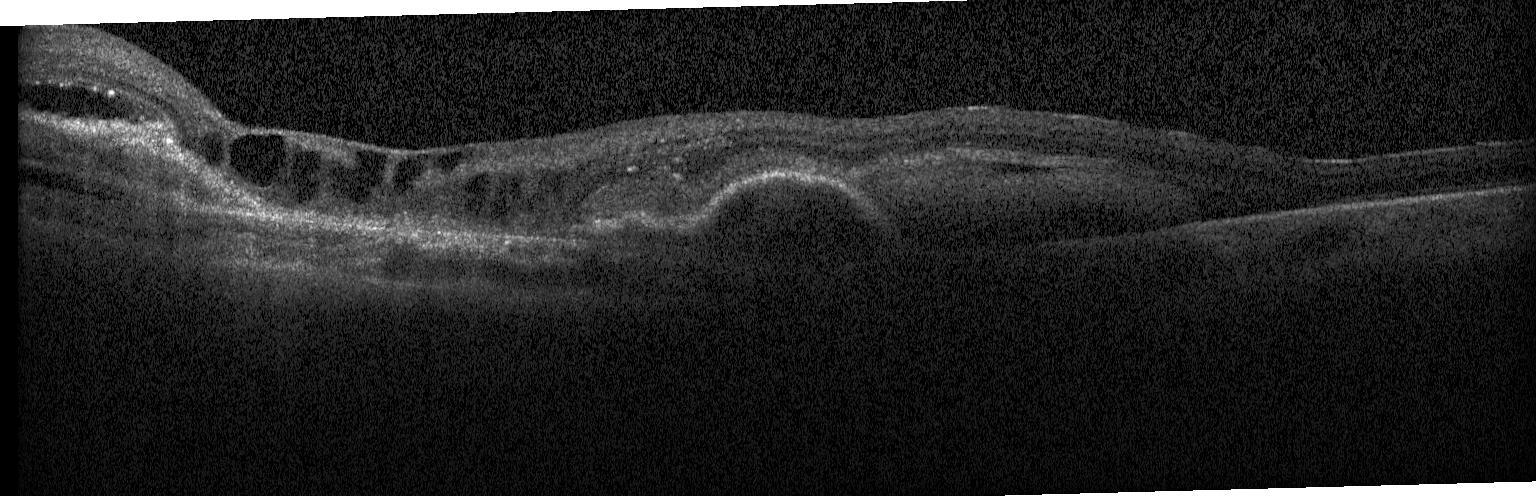
Optical coherence tomography B-scan
Finding: a choroidal neovascular membrane.